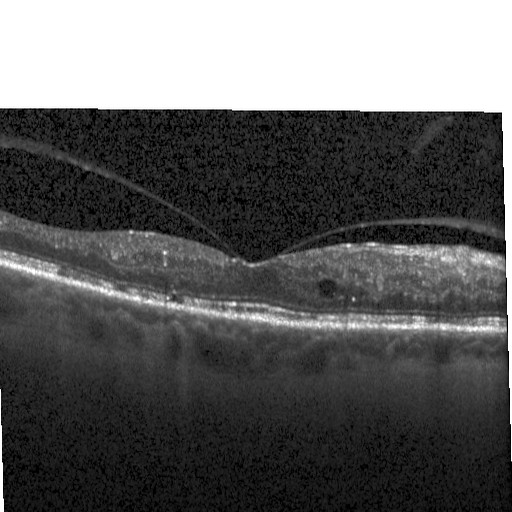
Finding: diabetic macular edema.